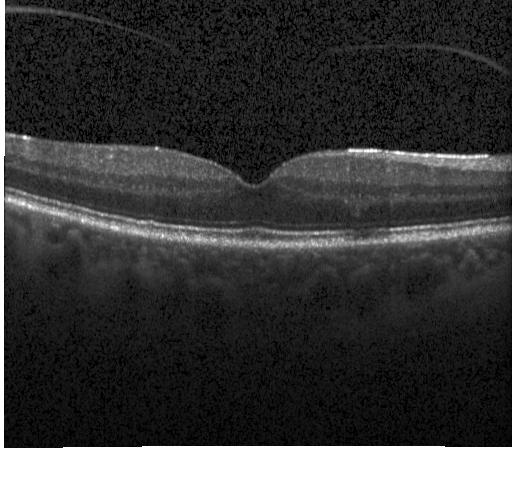 Acquired on a Heidelberg Spectralis. Centered on the fovea. OCT line scan. SD-OCT — Assessment: no choroidal neovascularization, diabetic macular edema, or drusen.